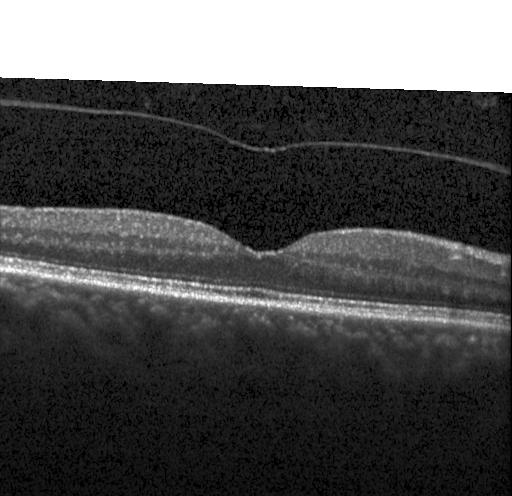
Spectral-domain OCT · optical coherence tomography B-scan. No choroidal neovascularization, no diabetic macular edema, and no drusen.